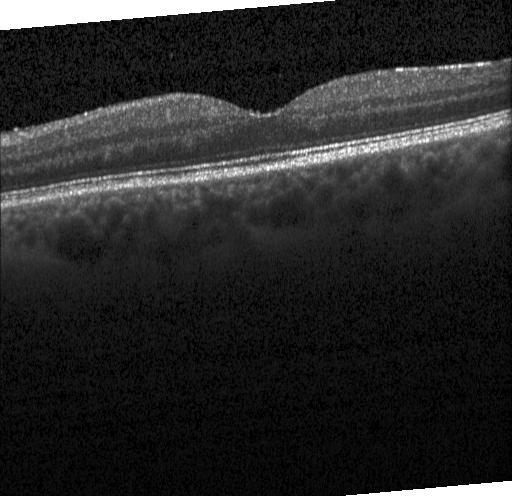
No evidence of choroidal neovascularization, diabetic macular edema, or drusen.